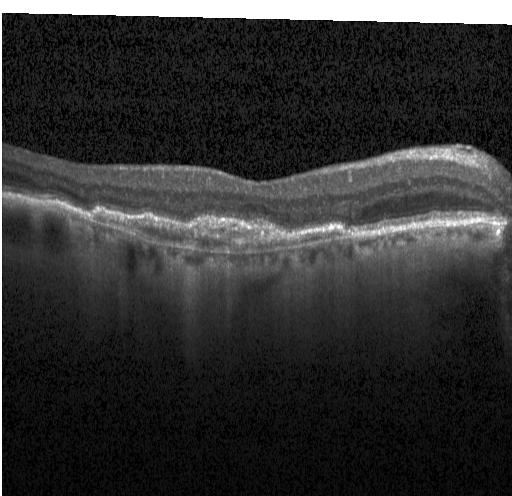

Macular OCT demonstrating a choroidal neovascular membrane.